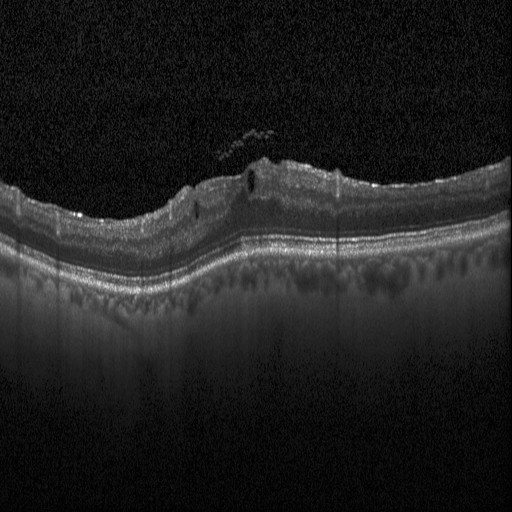 The scan shows DME.